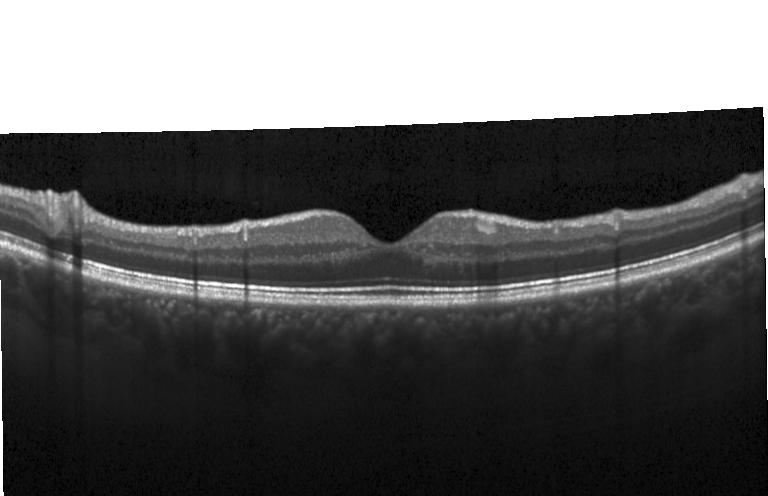 Instrument: Heidelberg Spectralis · optical coherence tomography B-scan · spectral-domain OCT · macular scan
Impression: no CNV, no DME, and no drusen.